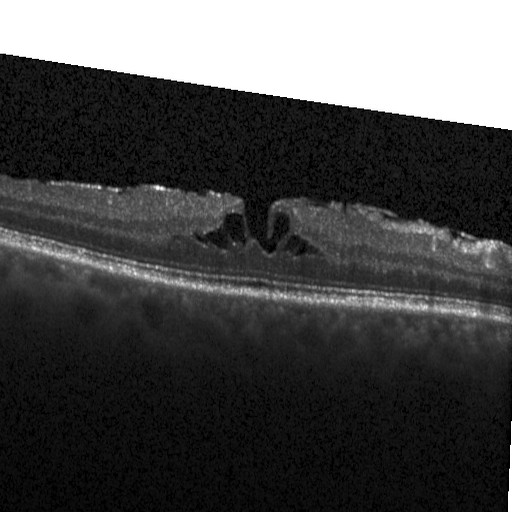
Horizontal scan through the fovea. Optical coherence tomography B-scan. SD-OCT. Instrument: Heidelberg Spectralis.
Finding: DME.